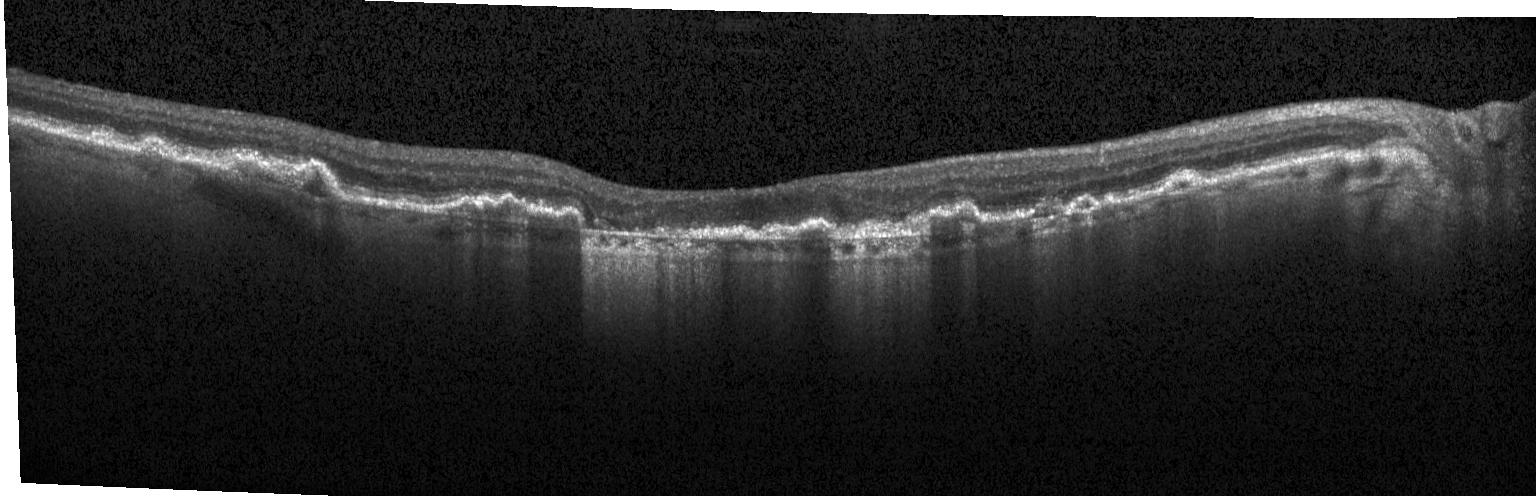

Centered on the fovea · optical coherence tomography scan
Impression: choroidal neovascularization.